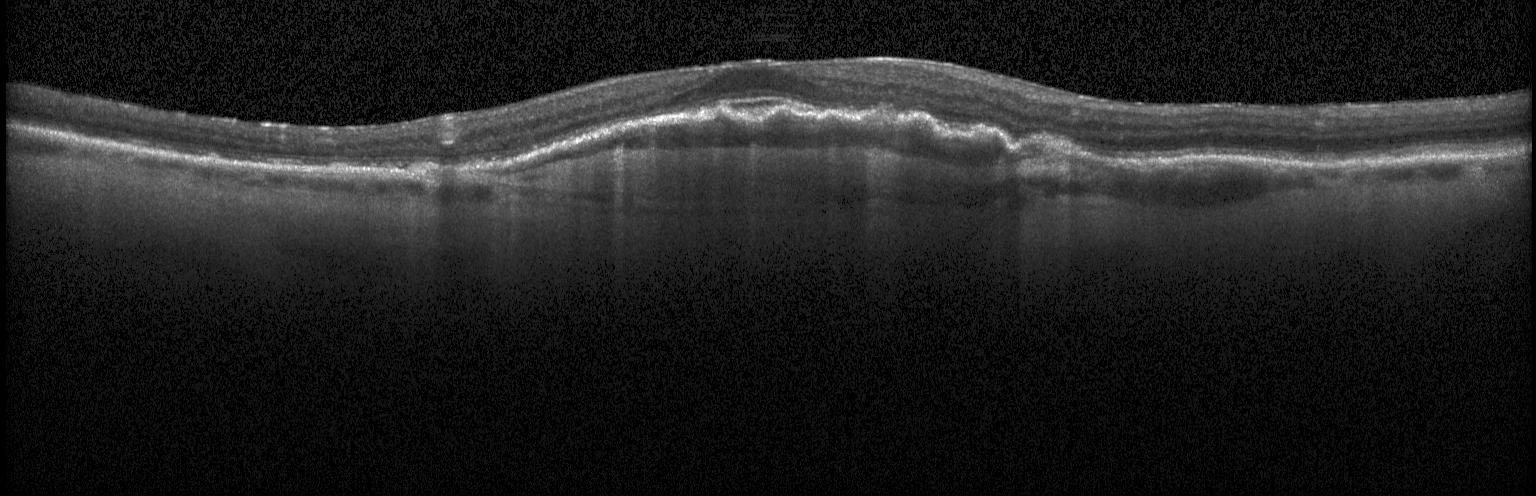 Instrument: Heidelberg Spectralis · spectral-domain optical coherence tomography · retinal OCT B-scan. Diagnosis: a choroidal neovascular membrane.